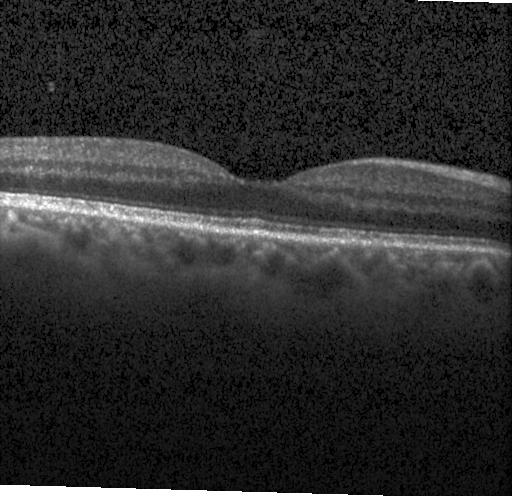

Optical coherence tomography scan, spectral-domain optical coherence tomography
This B-scan demonstrates neither choroidal neovascularization, diabetic macular edema, nor drusen.